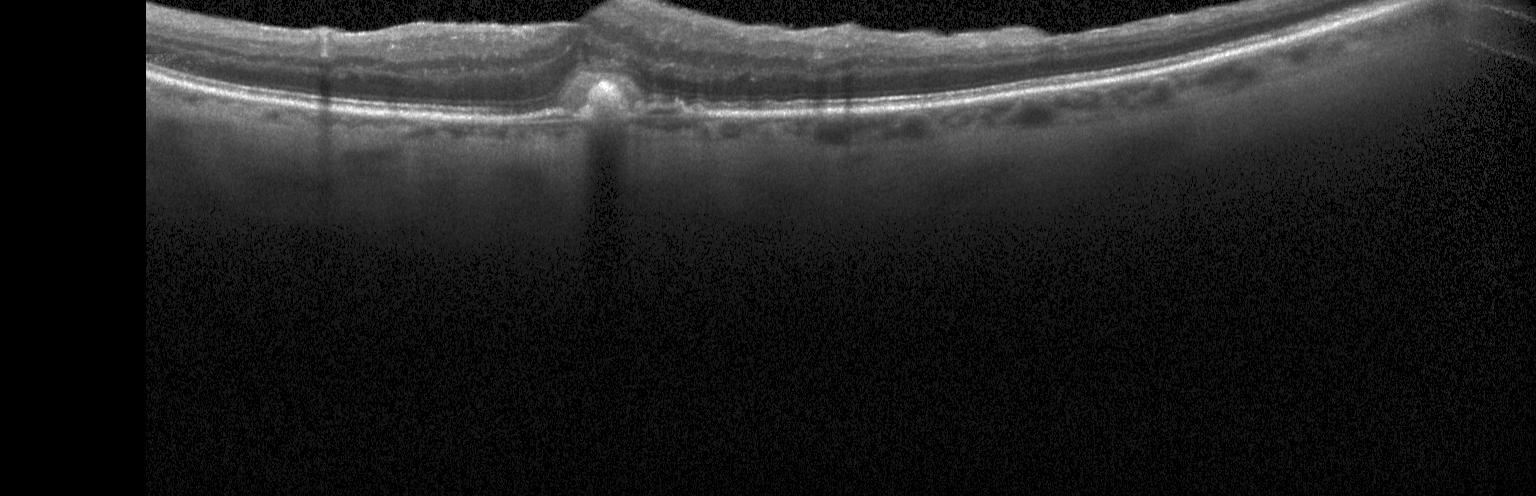 OCT finding: choroidal neovascularization (CNV).